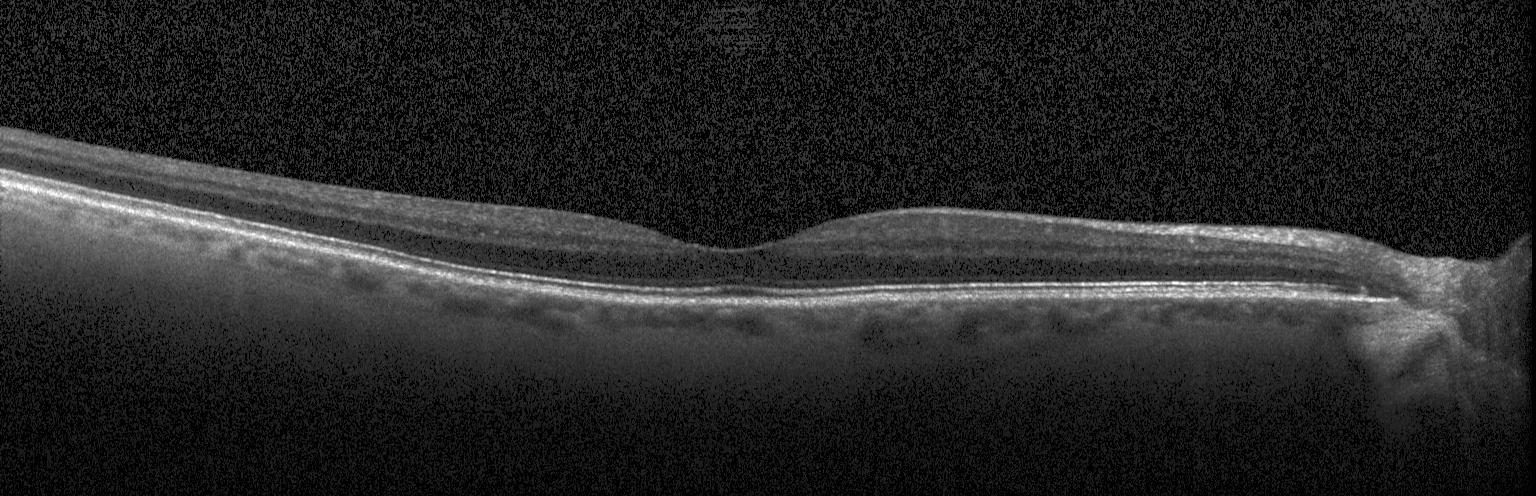

Impression: neither choroidal neovascularization, diabetic macular edema, nor drusen.